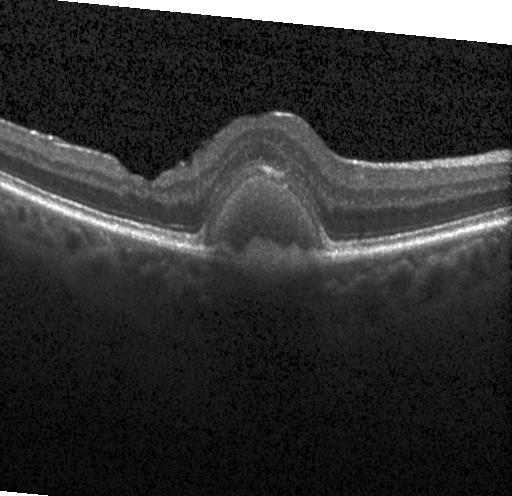 Horizontal scan through the fovea, optical coherence tomography scan, Heidelberg Spectralis OCT system, spectral-domain optical coherence tomography. Diagnosis: choroidal neovascularization.